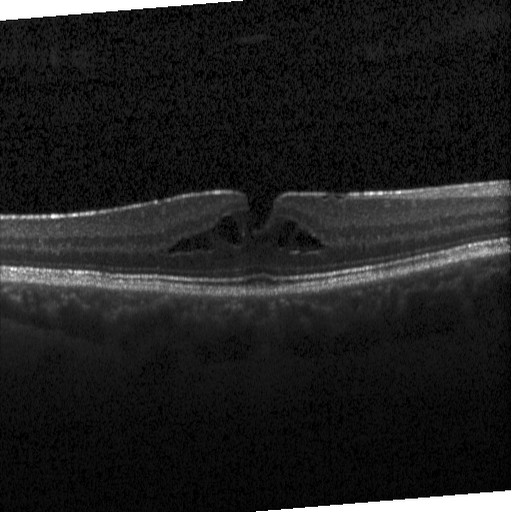 SD-OCT; horizontal scan through the fovea; optical coherence tomography scan — Impression: DME.